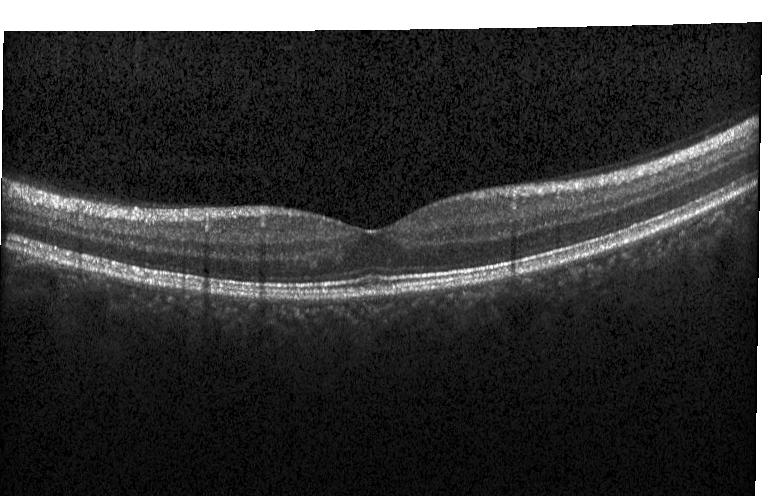
The scan shows neither choroidal neovascularization, diabetic macular edema, nor drusen.